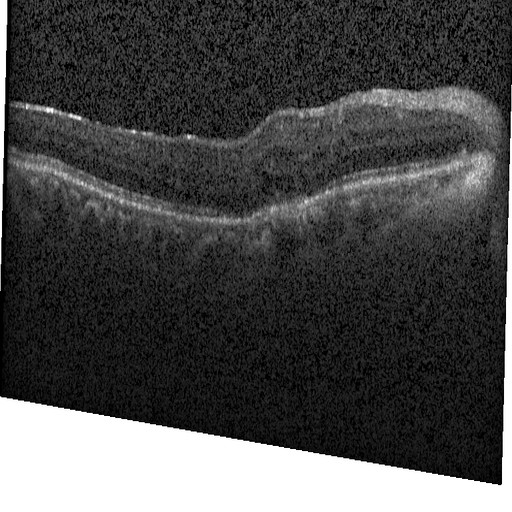 Optical coherence tomography scan — Diagnosis: diabetic macular edema.